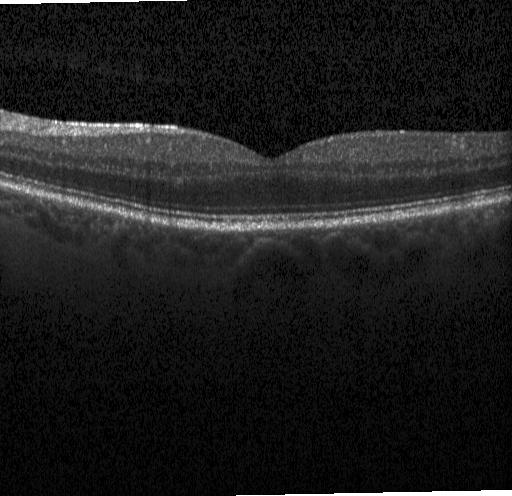
OCT B-scan
Impression: neither choroidal neovascularization, diabetic macular edema, nor drusen.